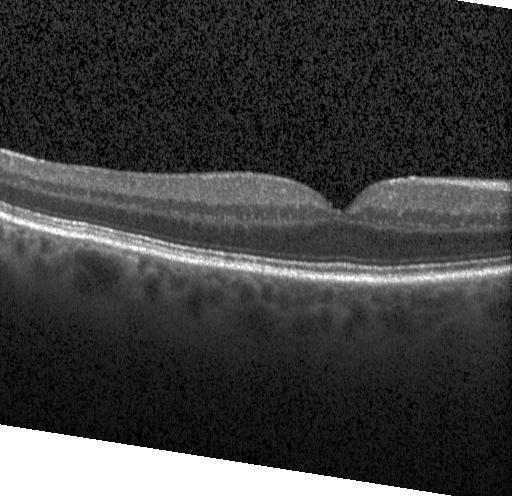
Spectral-domain OCT B-scan: neither CNV, DME, nor drusen.